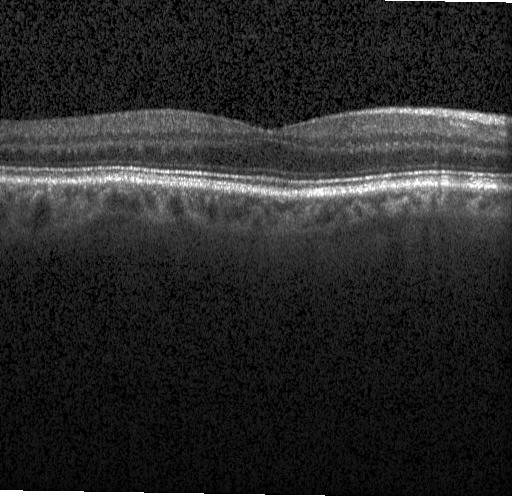

Finding: neither choroidal neovascularization, diabetic macular edema, nor drusen.